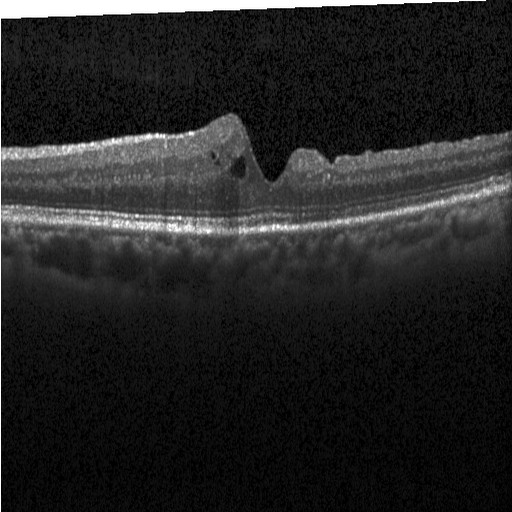 Fovea-centered. Optical coherence tomography B-scan. Acquired on a Heidelberg Spectralis. SD-OCT.
The scan shows diabetic macular edema (DME).